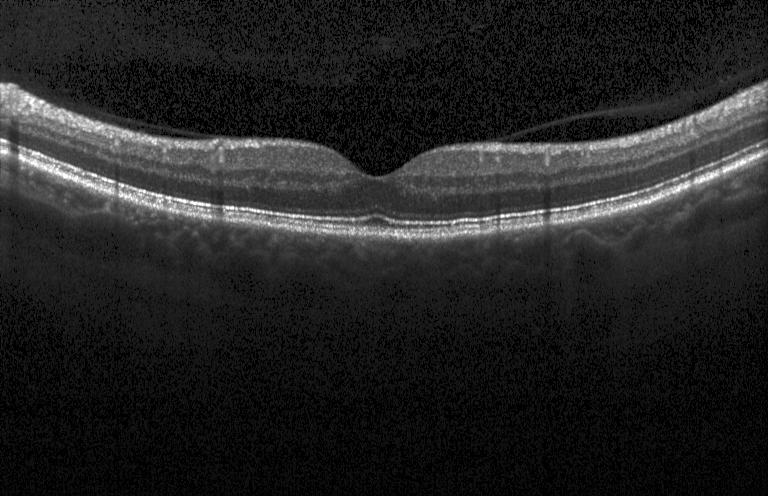 Through the macula · OCT line scan · Heidelberg Spectralis · spectral-domain OCT.
Impression: no CNV, no DME, and no drusen.